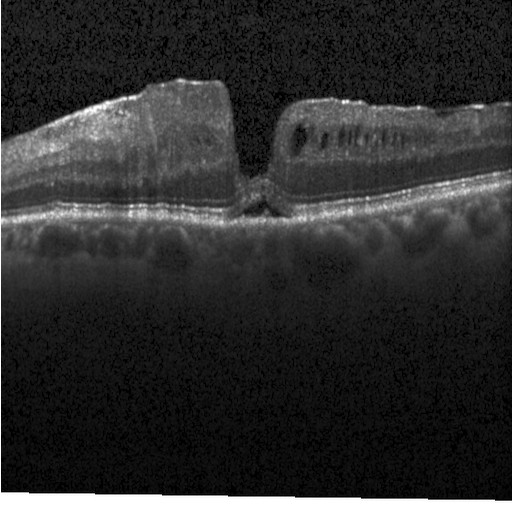
OCT line scan
The scan shows diabetic macular edema (DME).